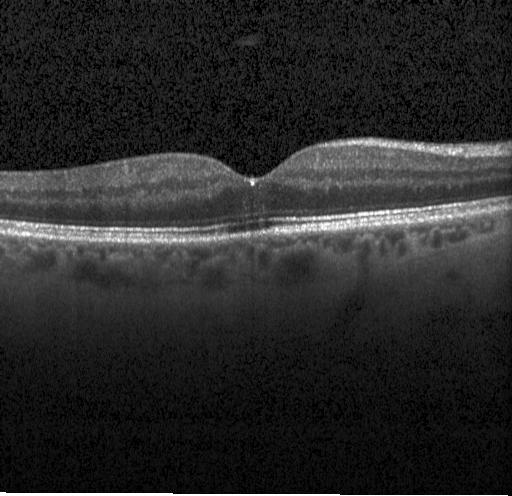
Dx: no evidence of choroidal neovascularization, diabetic macular edema, or drusen.